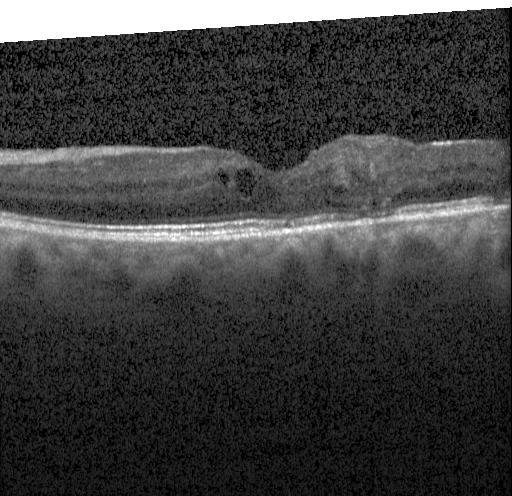 Retinal OCT B-scan
Macular OCT: diabetic macular edema (DME).